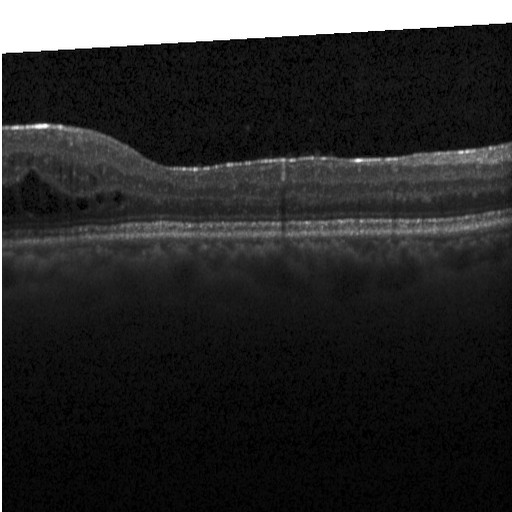

Macular OCT: diabetic macular edema.